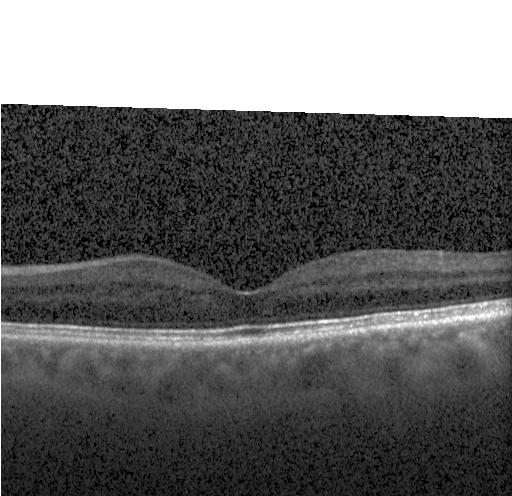 Spectral-domain OCT. Heidelberg Spectralis OCT system. OCT line scan.
The scan shows neither choroidal neovascularization, diabetic macular edema, nor drusen.